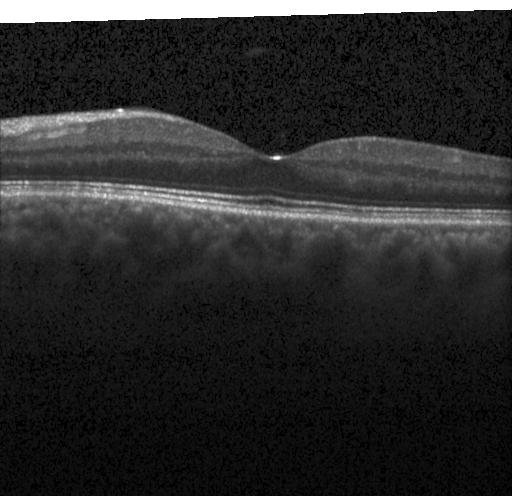
Optical coherence tomography B-scan. Instrument: Heidelberg Spectralis. Assessment: no choroidal neovascularization, no diabetic macular edema, and no drusen.